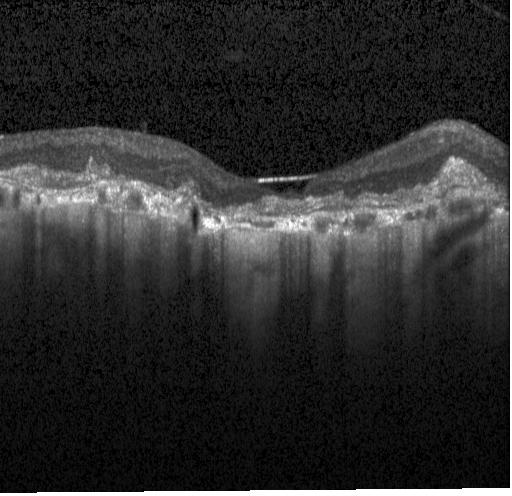 OCT B-scan showing choroidal neovascularization.